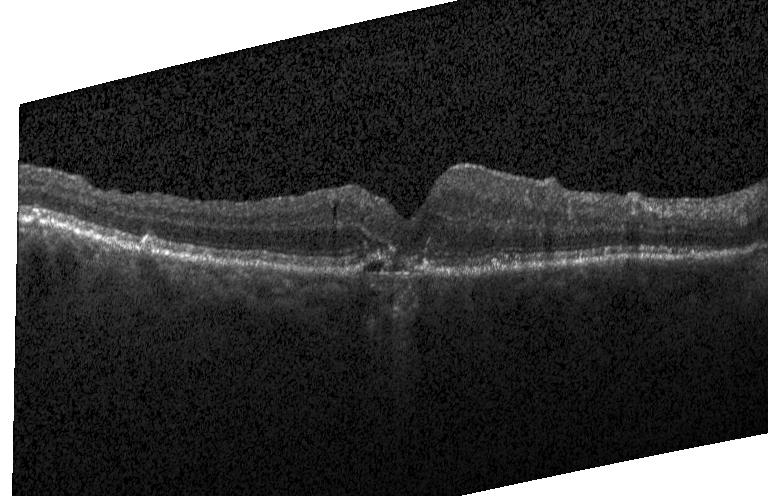 This B-scan demonstrates choroidal neovascularization.